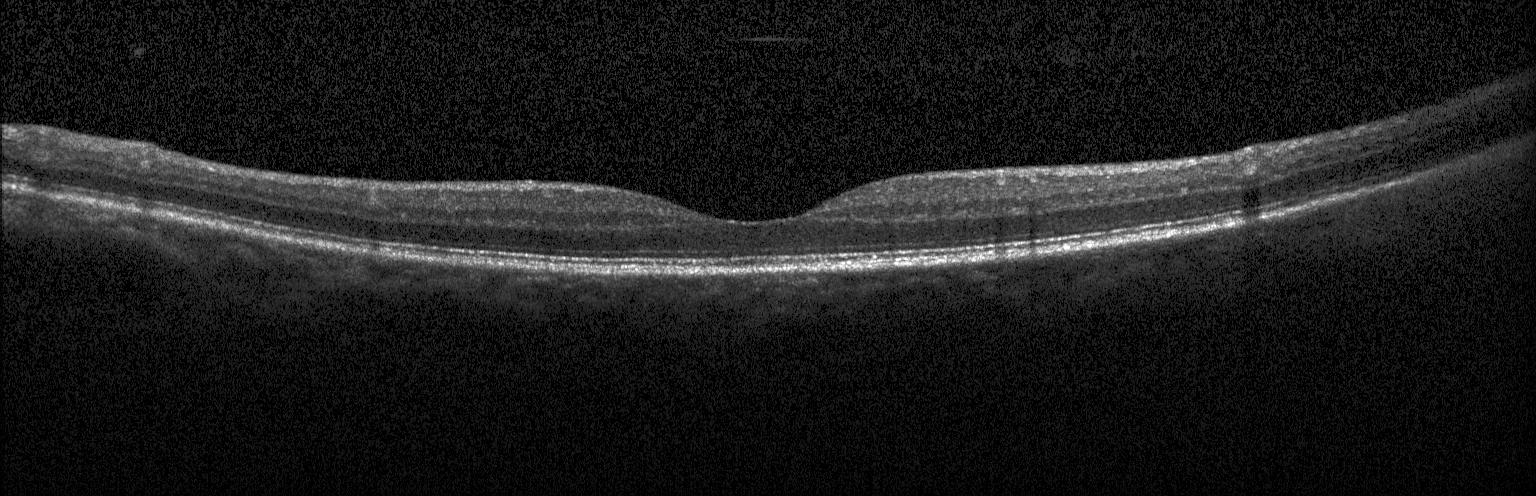
OCT B-scan — Finding: no CNV, DME, or drusen.